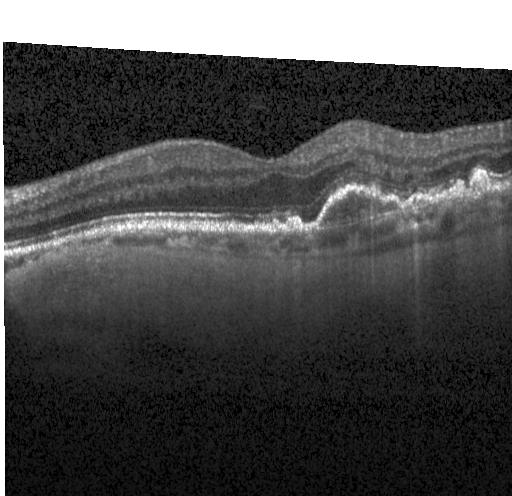
Horizontal scan through the fovea. Optical coherence tomography scan. Heidelberg Spectralis. Diagnosis: CNV.